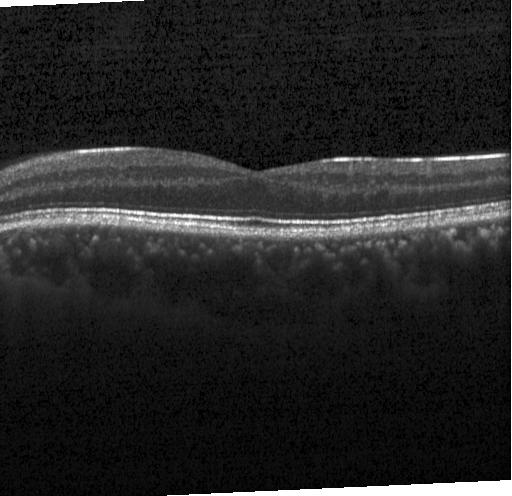 OCT B-scan showing no choroidal neovascularization, no diabetic macular edema, and no drusen.